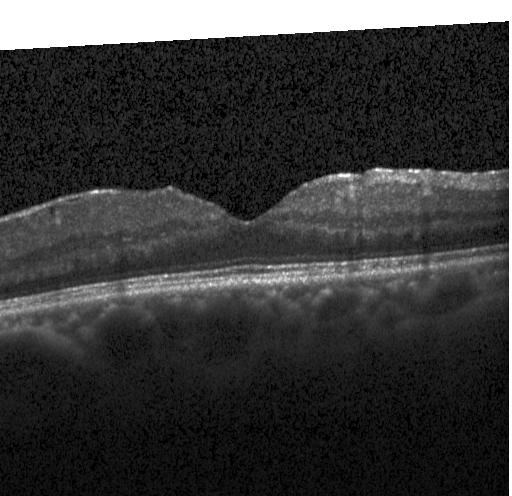
OCT B-scan showing neither CNV, DME, nor drusen.